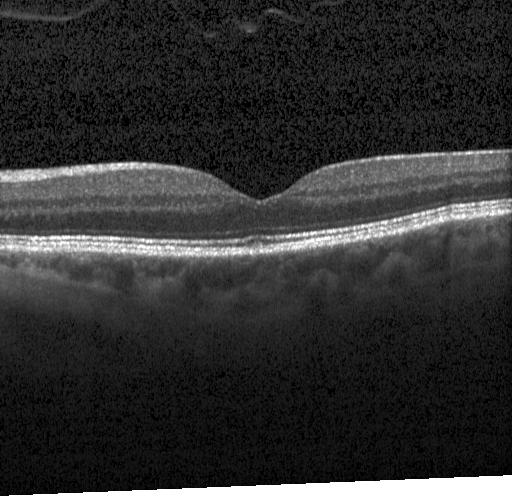
Retinal OCT cross-section. The scan shows no evidence of CNV, DME, or drusen.